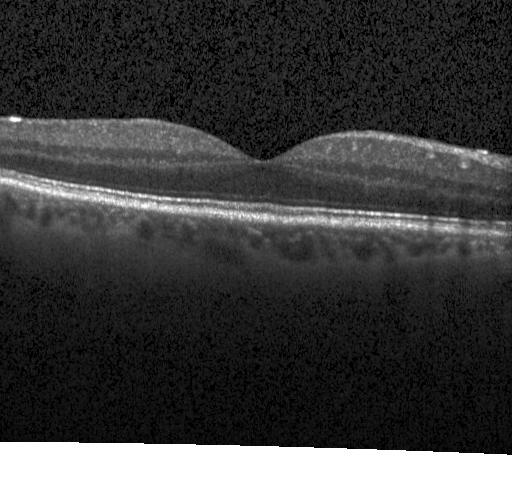 OCT finding: no choroidal neovascularization, no diabetic macular edema, and no drusen.